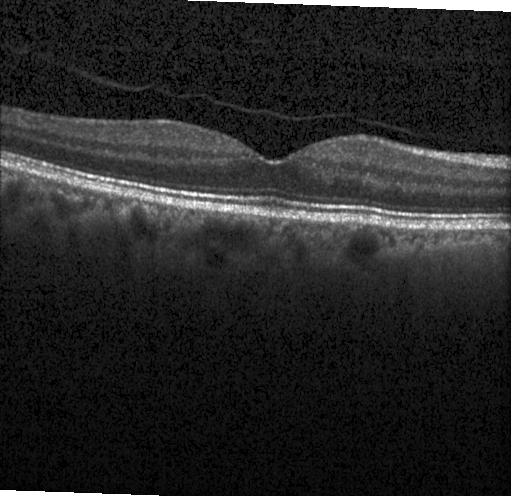
Acquired on a Heidelberg Spectralis, optical coherence tomography scan — Impression: no evidence of choroidal neovascularization, diabetic macular edema, or drusen.